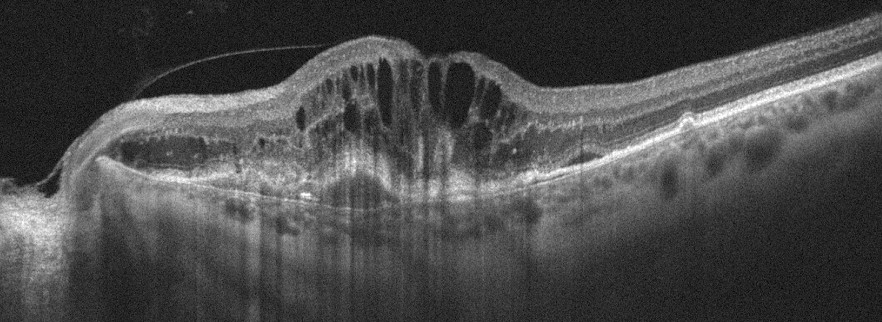

Retinal OCT B-scan; left eye.
Impression: age-related macular degeneration (AMD).